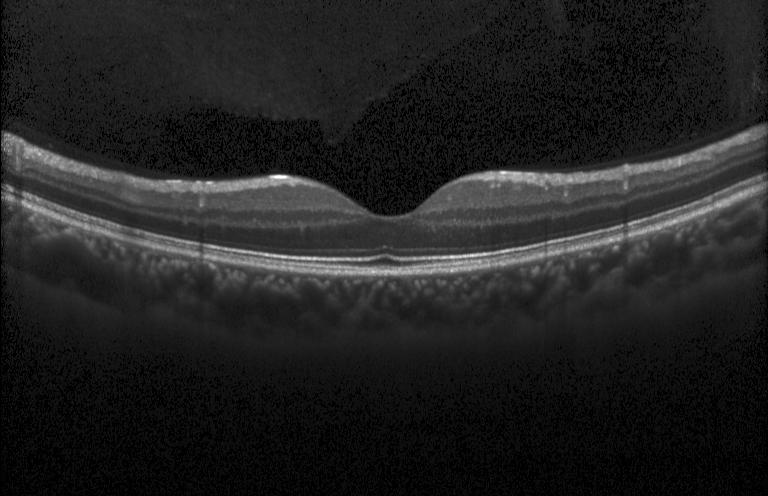 Macular OCT: no evidence of CNV, DME, or drusen.